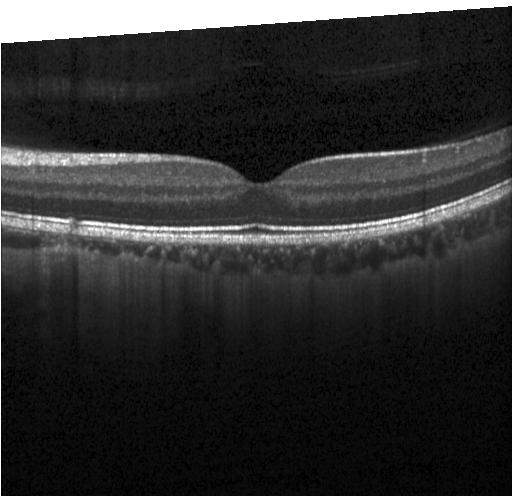

Macular OCT: no choroidal neovascularization, diabetic macular edema, or drusen.